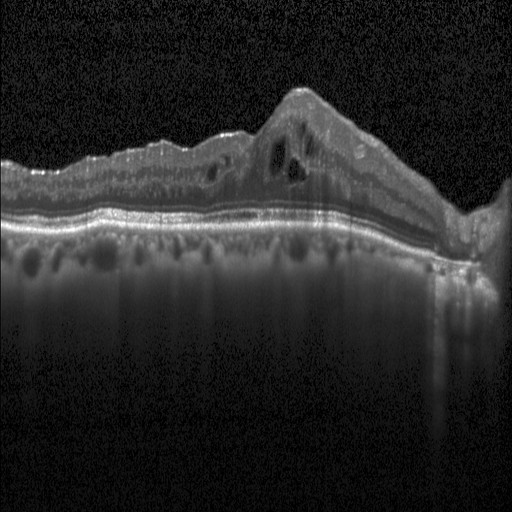

OCT B-scan. Acquired on a Heidelberg Spectralis. SD-OCT
Dx: diabetic macular edema.